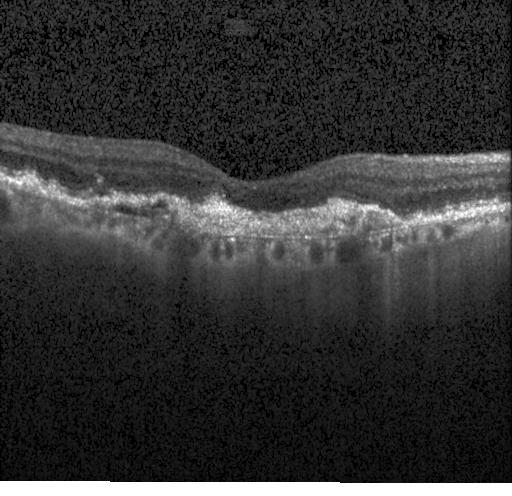 Assessment: a choroidal neovascular membrane.